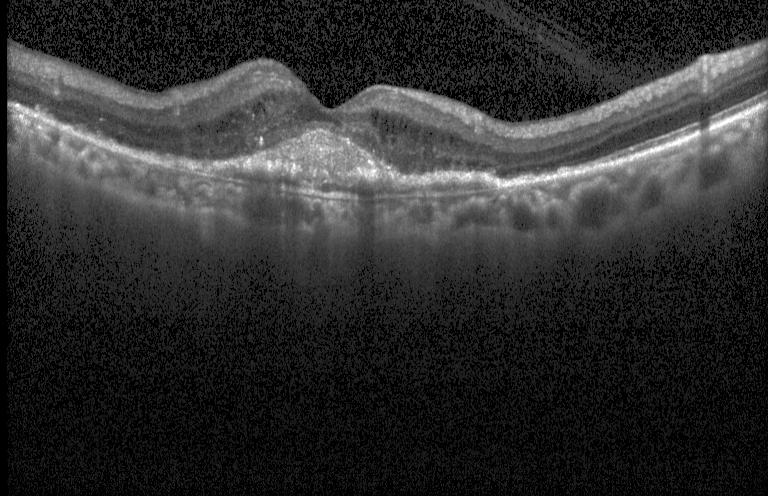
Macular OCT demonstrating a choroidal neovascular membrane.